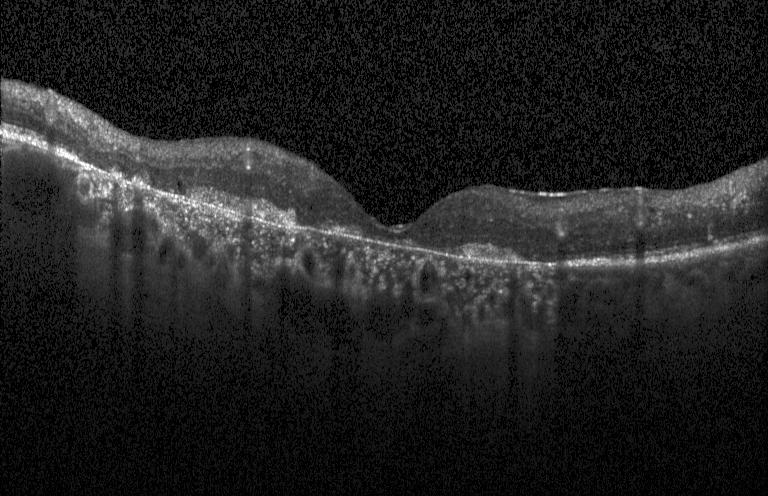

OCT line scan; Heidelberg Spectralis
Macular OCT: CNV.